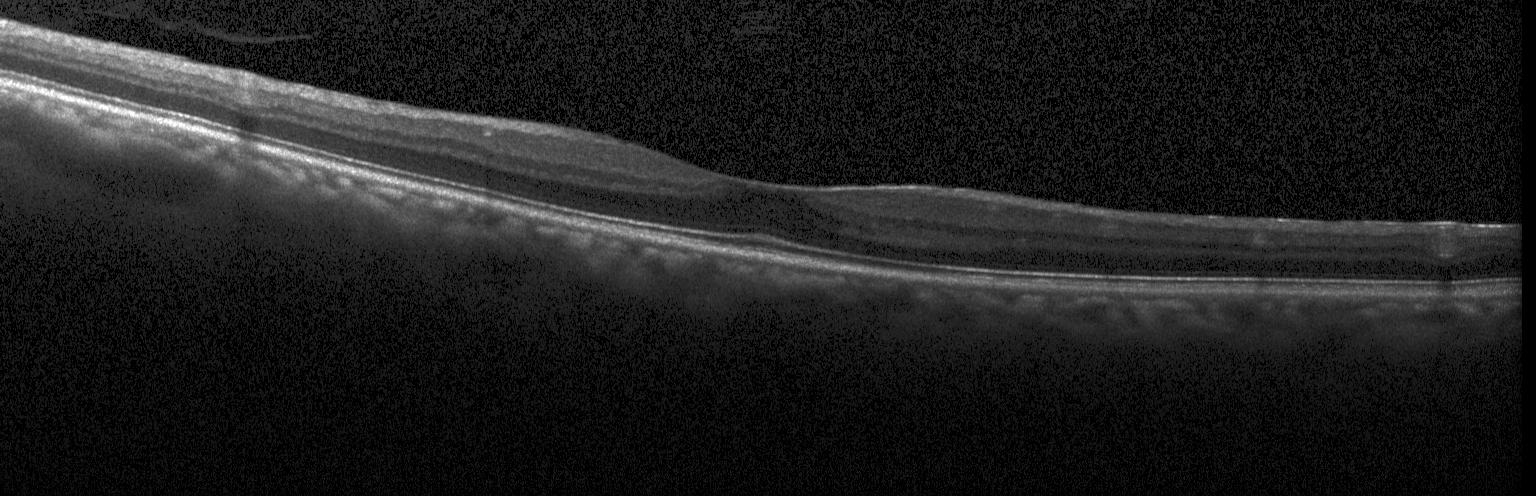

Spectral-domain optical coherence tomography; Heidelberg Spectralis OCT system; retinal OCT B-scan; centered on the fovea. The scan shows no choroidal neovascularization, diabetic macular edema, or drusen.